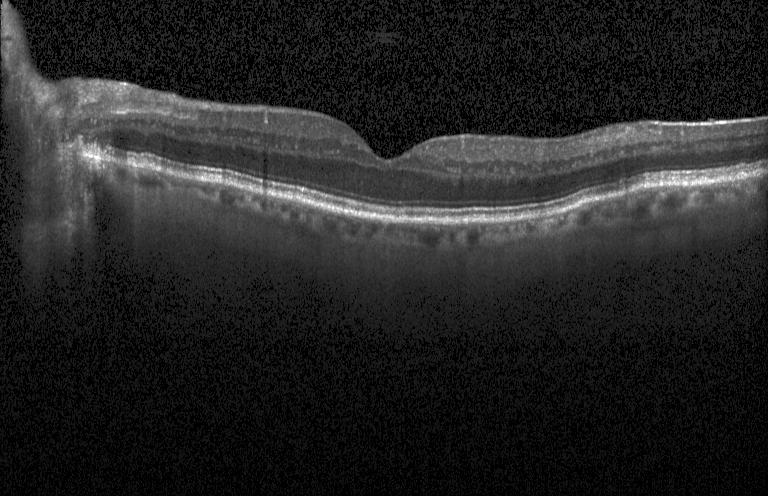
OCT line scan.
The scan shows no choroidal neovascularization, diabetic macular edema, or drusen.